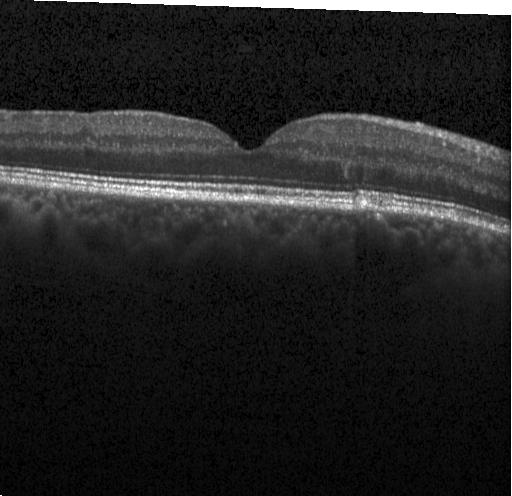
Acquired on a Heidelberg Spectralis, retinal OCT cross-section
Impression: neither choroidal neovascularization, diabetic macular edema, nor drusen.